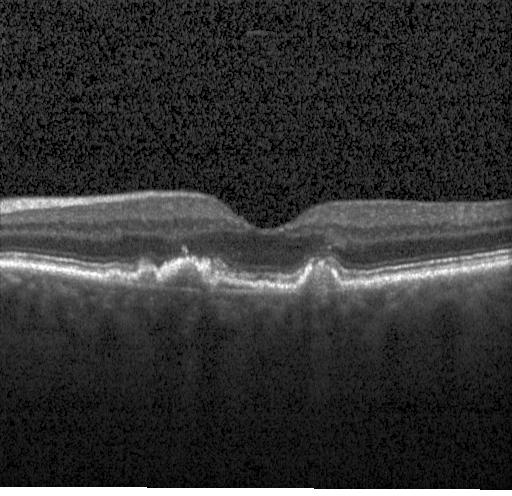

Heidelberg Spectralis OCT system, spectral-domain optical coherence tomography, retinal OCT cross-section, centered on the fovea — Finding: CNV.